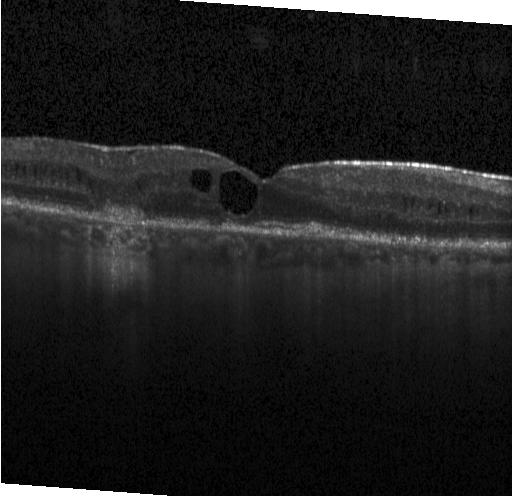

Retinal OCT cross-section · acquired on a Heidelberg Spectralis
Diagnosis: choroidal neovascularization (CNV).